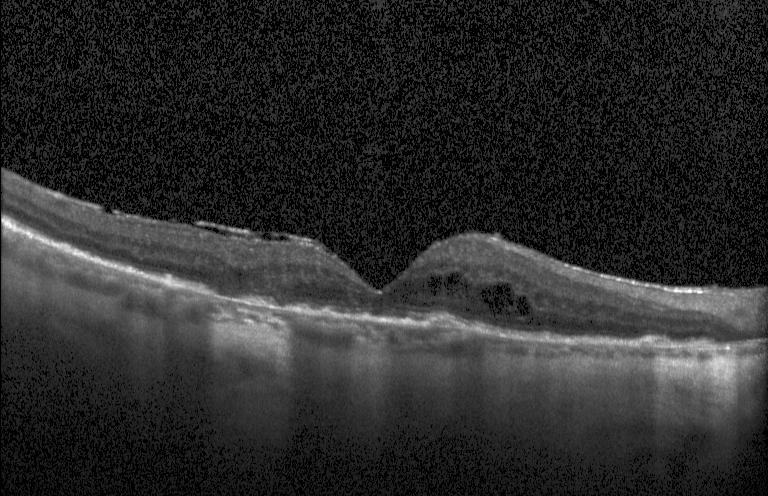
SD-OCT; instrument: Heidelberg Spectralis; retinal OCT cross-section — This B-scan demonstrates DME.